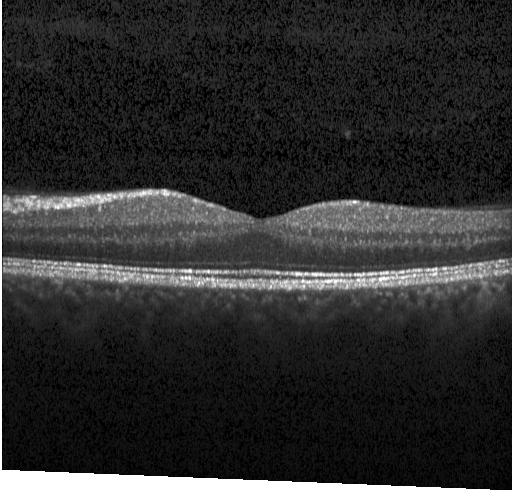
OCT B-scan showing no evidence of CNV, DME, or drusen.